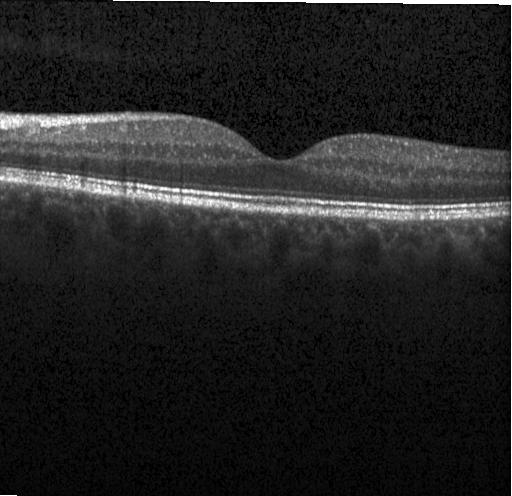

The scan shows no evidence of CNV, DME, or drusen.